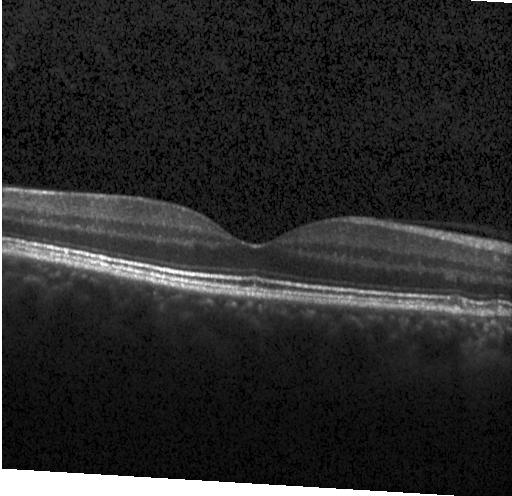
Dx: no CNV, no DME, and no drusen.